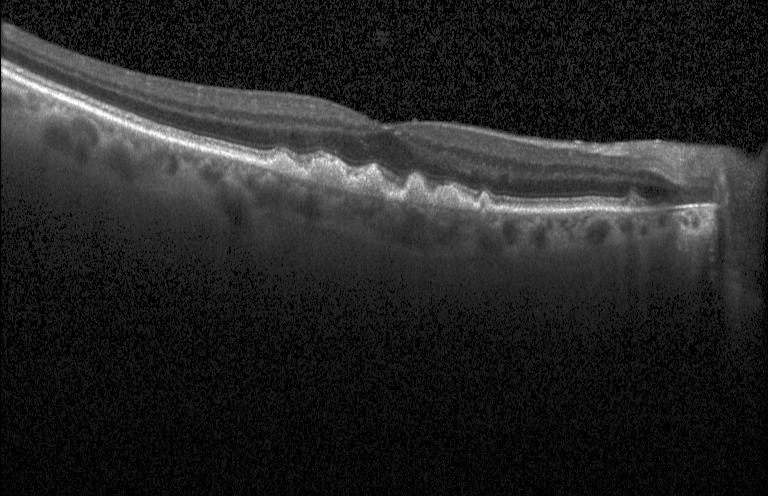
Spectral-domain OCT B-scan: multiple drusen.